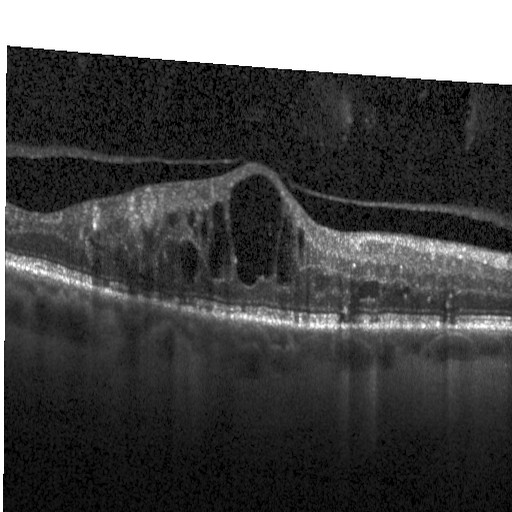

Dx: diabetic macular edema.